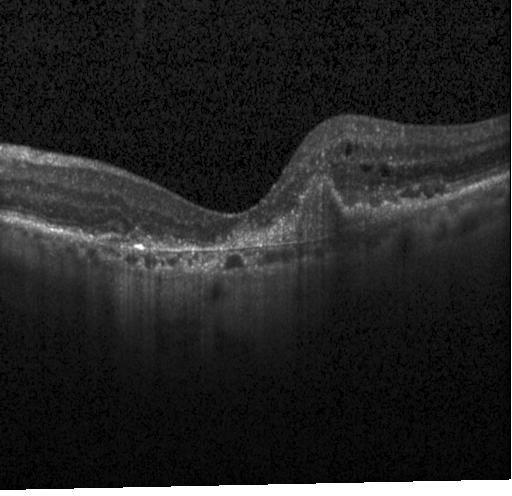 OCT B-scan.
Impression: choroidal neovascularization (CNV).